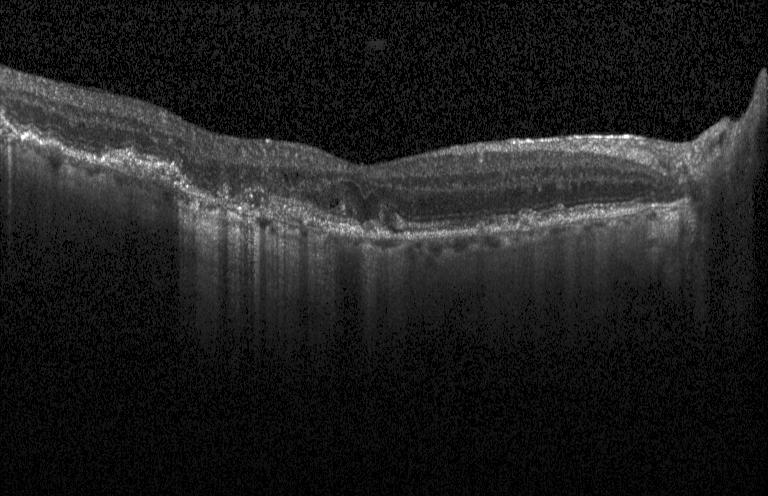
Assessment: choroidal neovascularization.